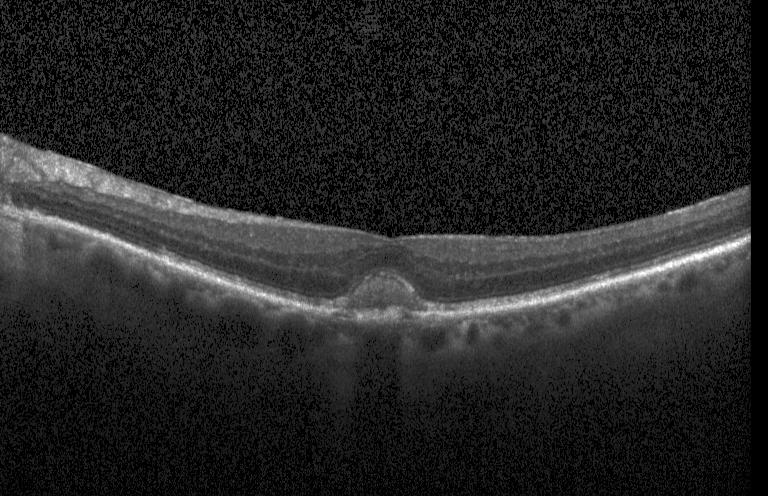

OCT B-scan. Finding: choroidal neovascularization.